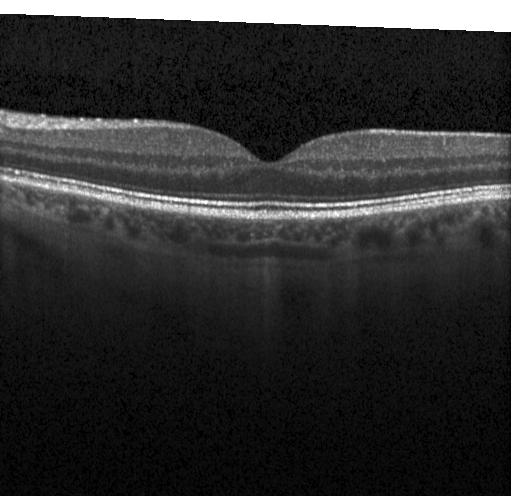
Assessment: no choroidal neovascularization, diabetic macular edema, or drusen.